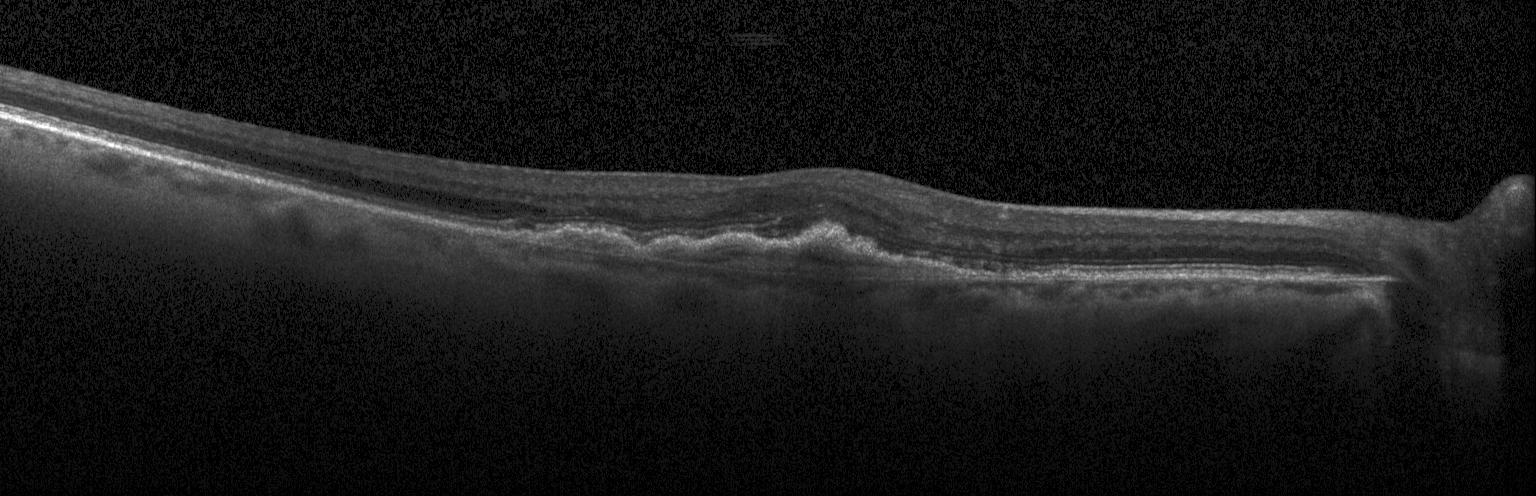

Macular OCT: choroidal neovascularization (CNV).